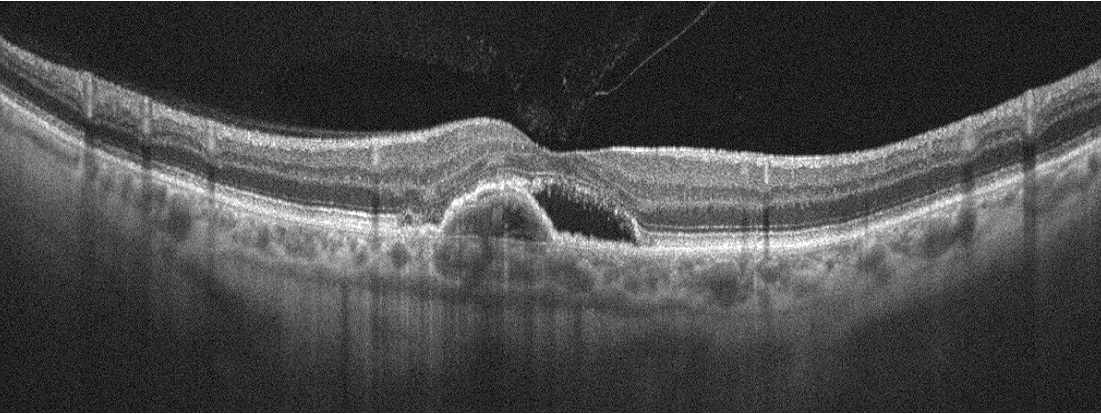 Retinal OCT cross-section, macular scan — Diagnosis: age-related macular degeneration.